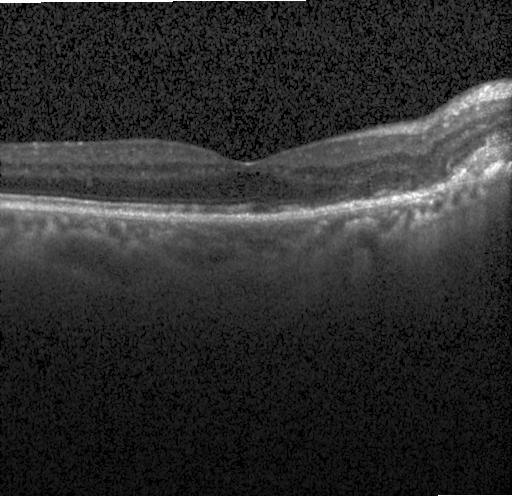

Dx: a choroidal neovascular membrane.